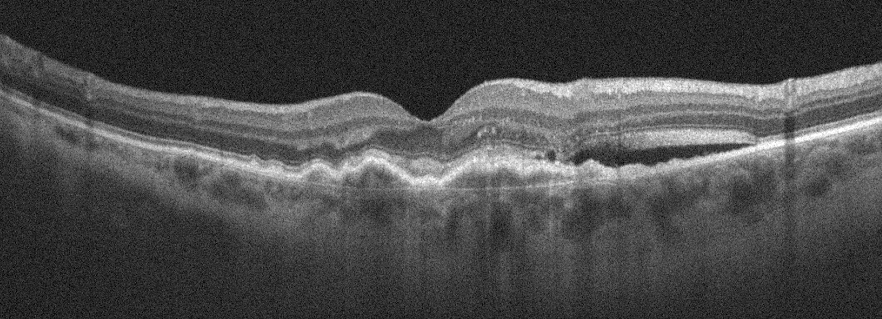
OS. Macular scan. Acquired on an Optovue Avanti RTVue XR. Optical coherence tomography B-scan. Diagnosis: age-related macular degeneration (AMD).